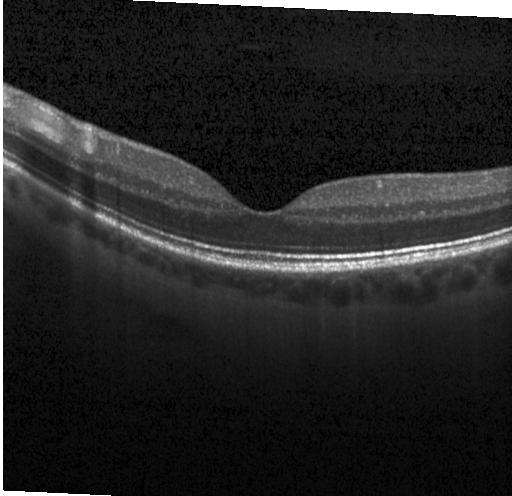 Spectral-domain OCT B-scan: neither choroidal neovascularization, diabetic macular edema, nor drusen.